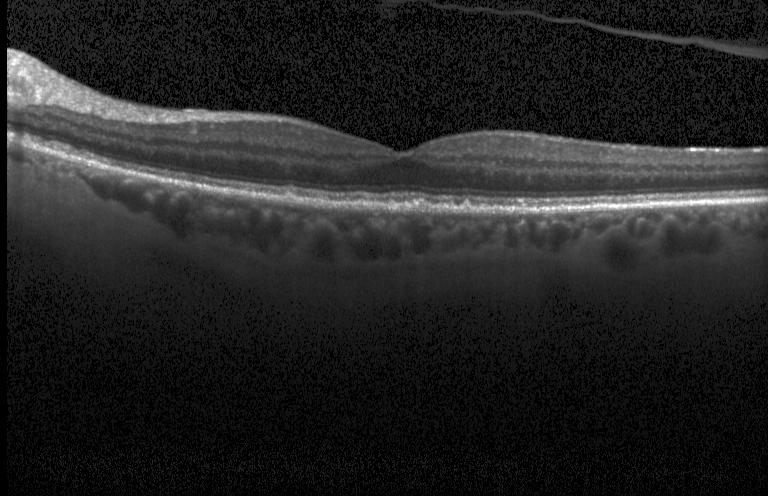
This B-scan demonstrates multiple drusen.